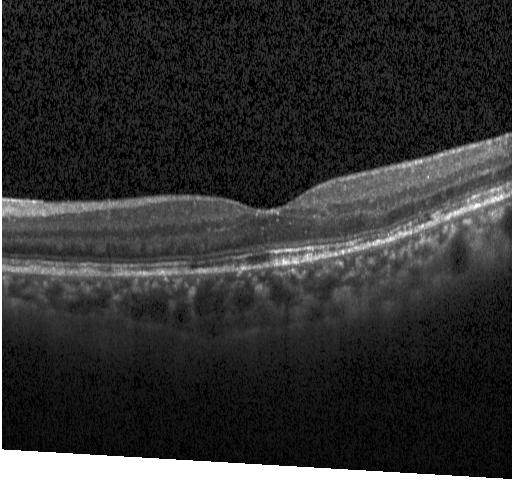 OCT finding: no choroidal neovascularization, diabetic macular edema, or drusen.